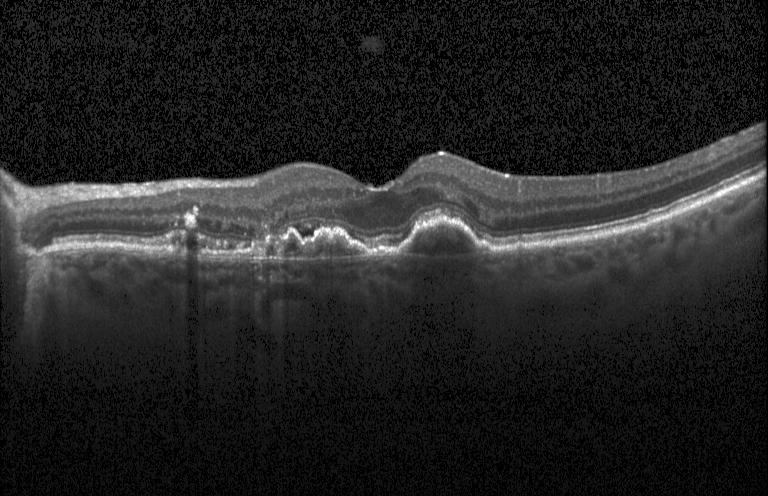
Retinal OCT cross-section showing a choroidal neovascular membrane.